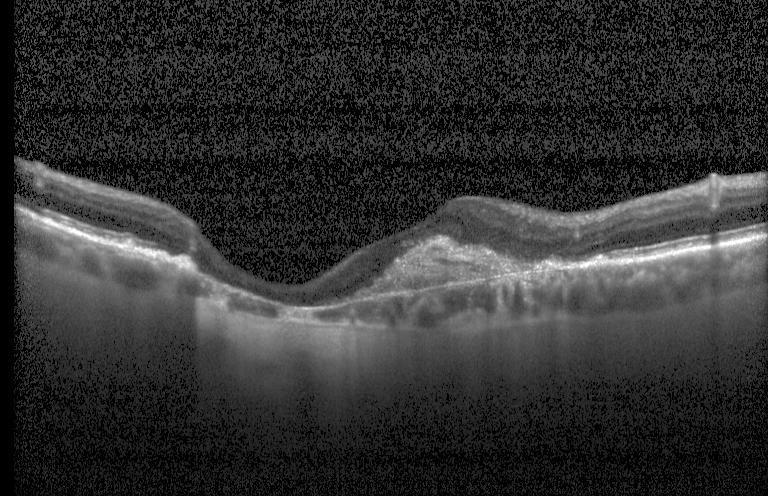

Dx: choroidal neovascularization (CNV).